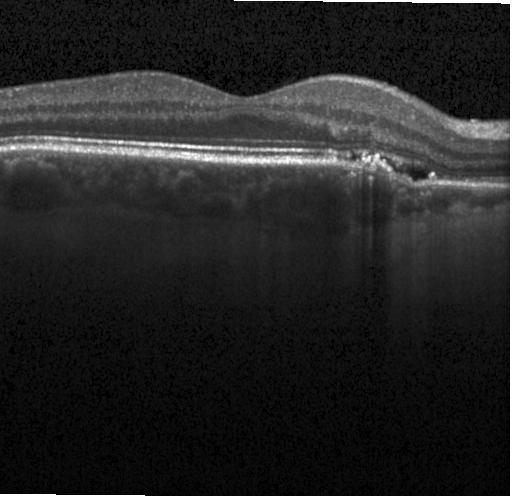

OCT line scan; horizontal scan through the fovea; SD-OCT; instrument: Heidelberg Spectralis — This B-scan demonstrates a choroidal neovascular membrane.